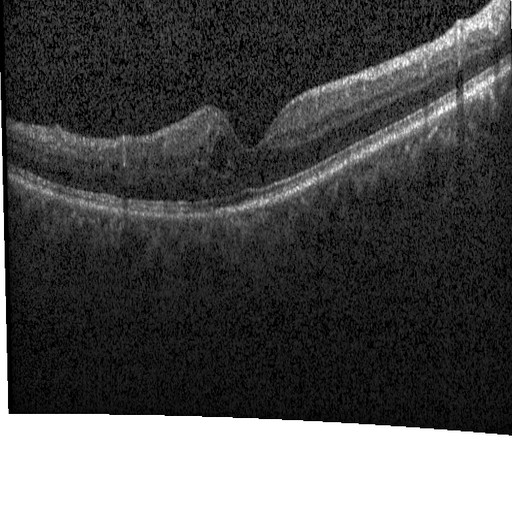
Acquired on a Heidelberg Spectralis, retinal OCT B-scan, centered on the fovea, spectral-domain optical coherence tomography — Finding: DME.